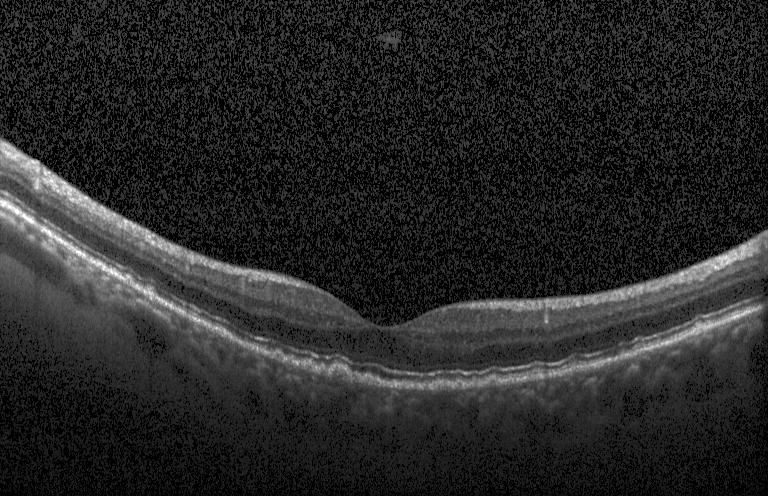 Diagnosis: drusen.